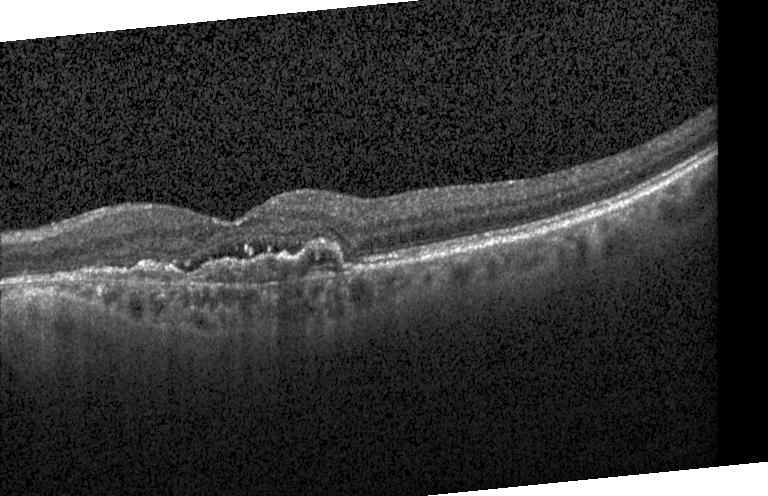
Optical coherence tomography scan. CNV.